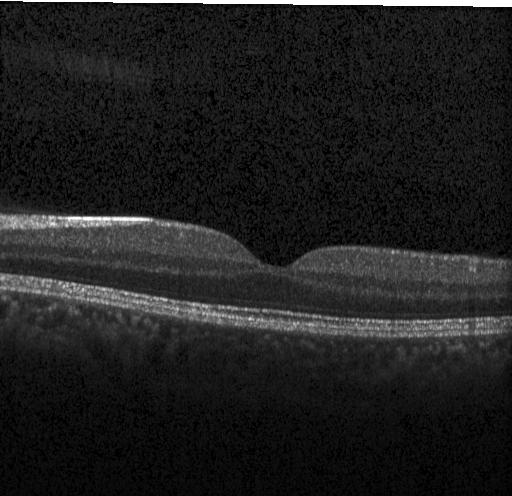
OCT B-scan.
This B-scan demonstrates no evidence of choroidal neovascularization, diabetic macular edema, or drusen.